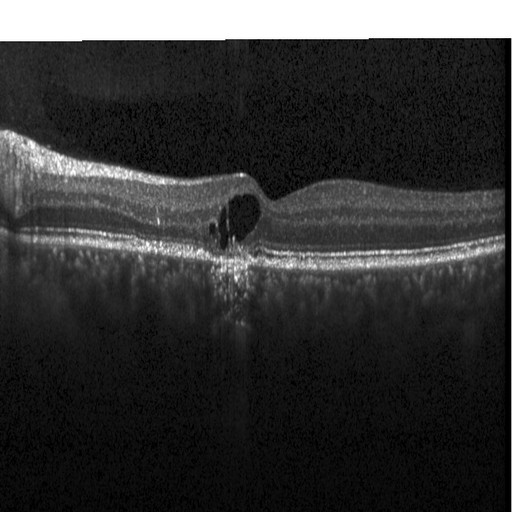

Optical coherence tomography B-scan, instrument: Heidelberg Spectralis, spectral-domain OCT, through the macula. This B-scan demonstrates diabetic macular edema.